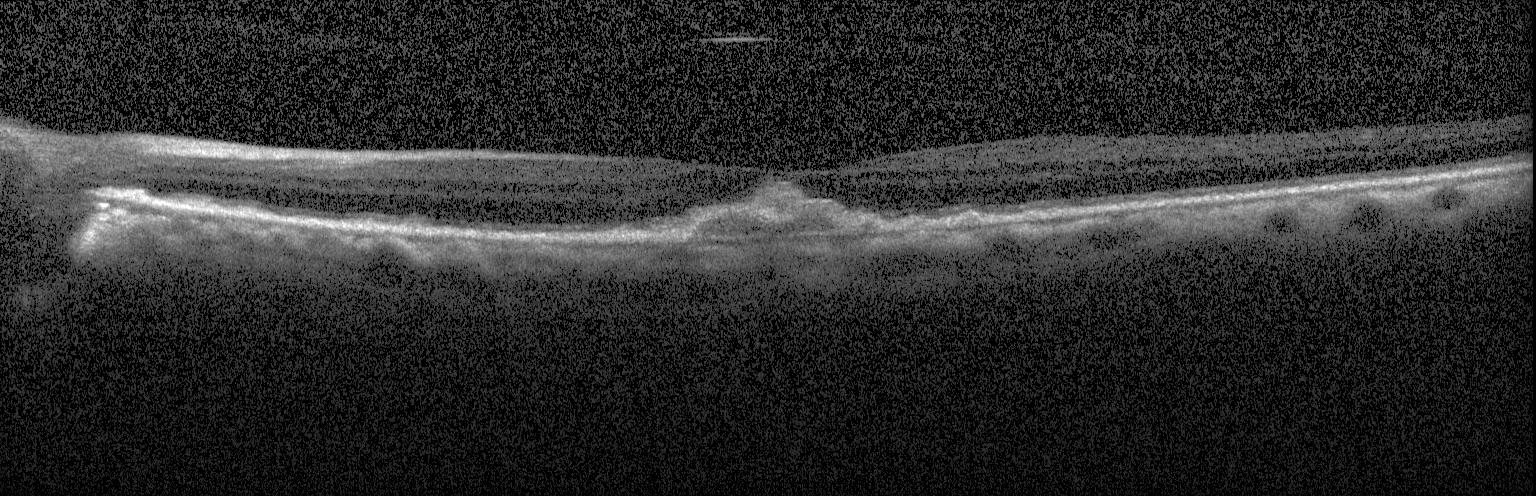

Diagnosis: a choroidal neovascular membrane.